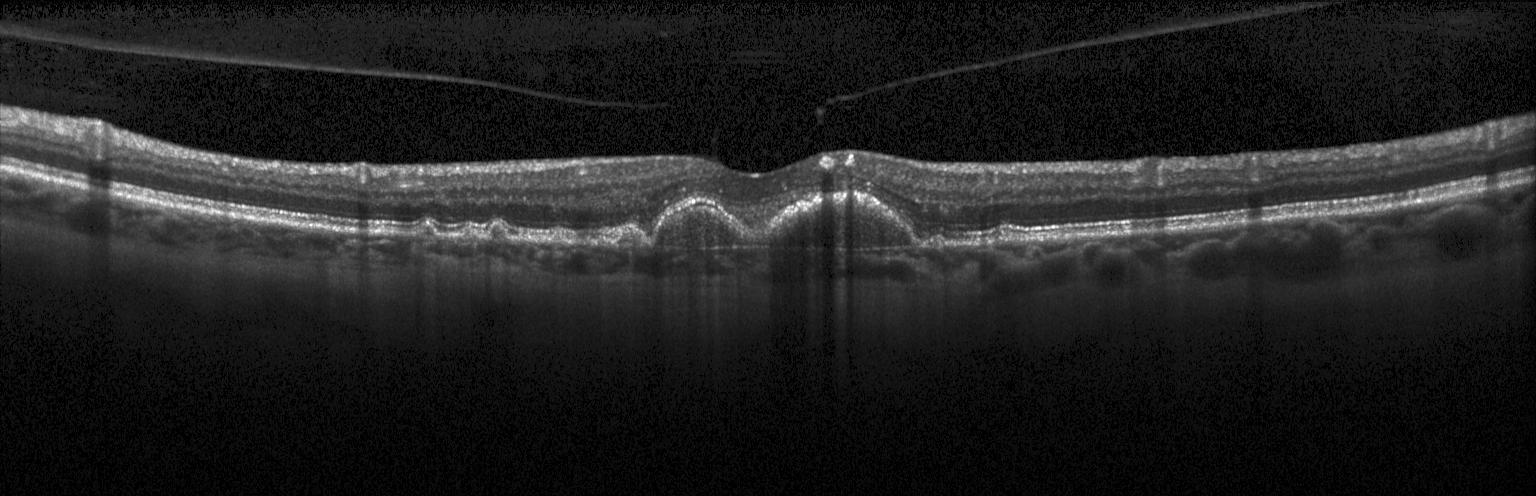

The scan shows choroidal neovascularization (CNV).